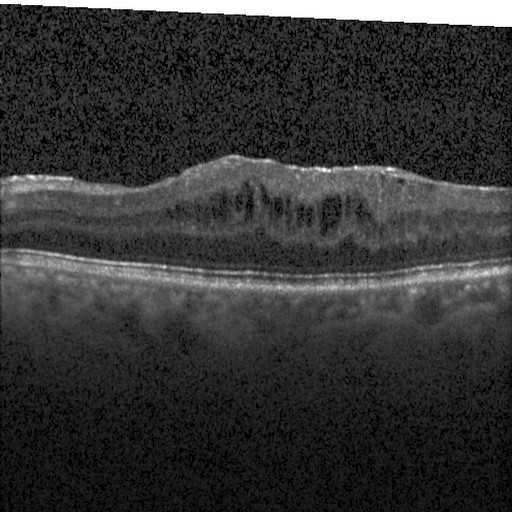
SD-OCT, retinal OCT cross-section. Finding: diabetic macular edema (DME).